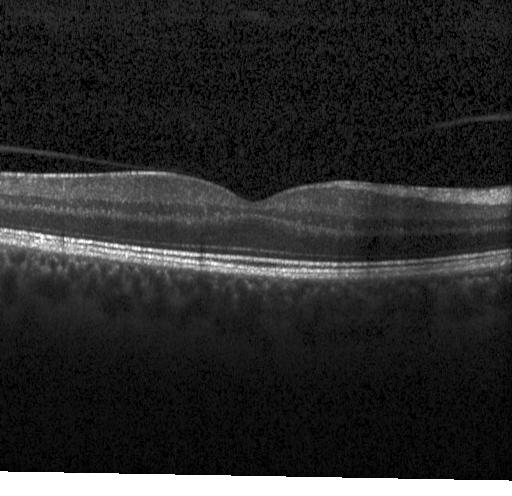 Assessment: no CNV, DME, or drusen.